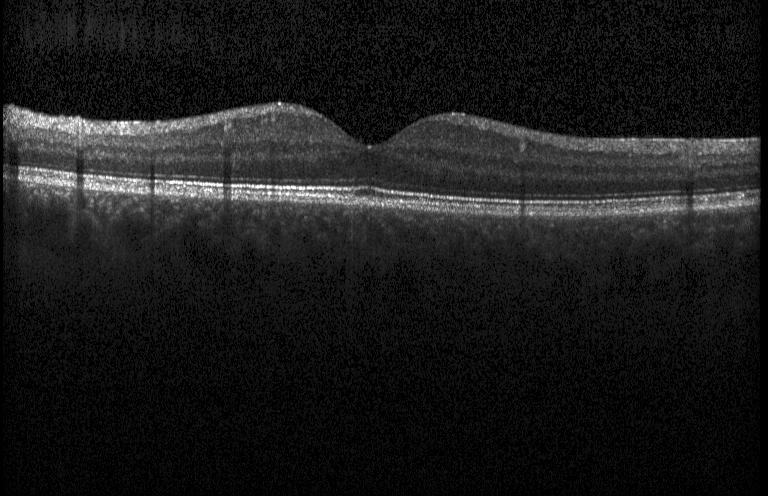 Retinal OCT cross-section showing no evidence of choroidal neovascularization, diabetic macular edema, or drusen.